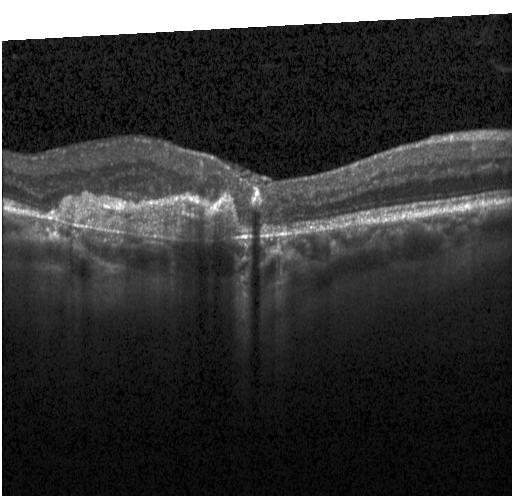 Spectral-domain optical coherence tomography, optical coherence tomography scan. Macular OCT: a choroidal neovascular membrane.